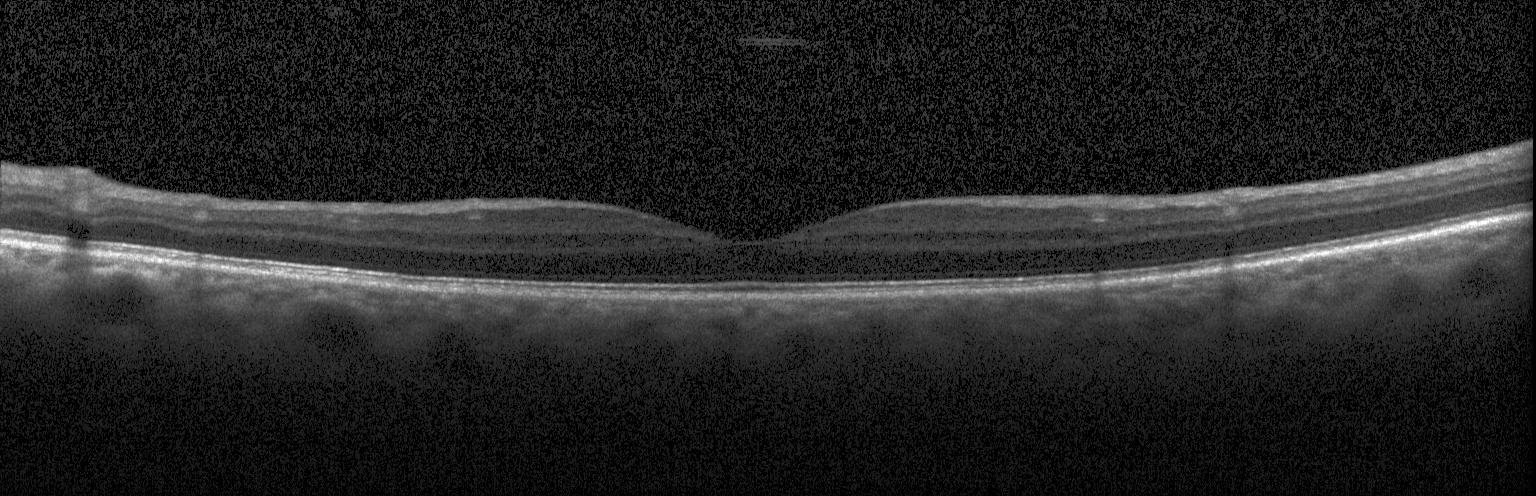

OCT B-scan showing no CNV, DME, or drusen.